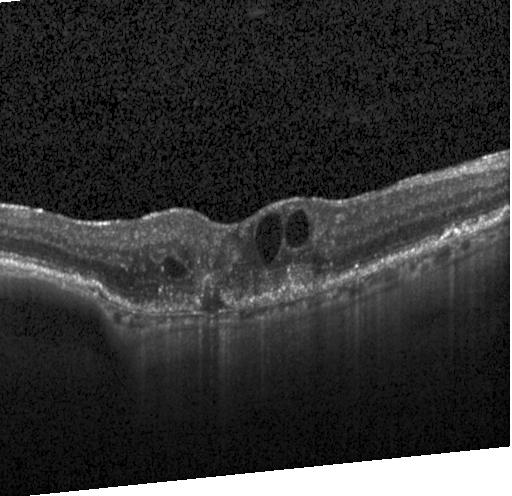
SD-OCT. Acquired on a Heidelberg Spectralis. OCT line scan. Centered on the fovea
This B-scan demonstrates a choroidal neovascular membrane.